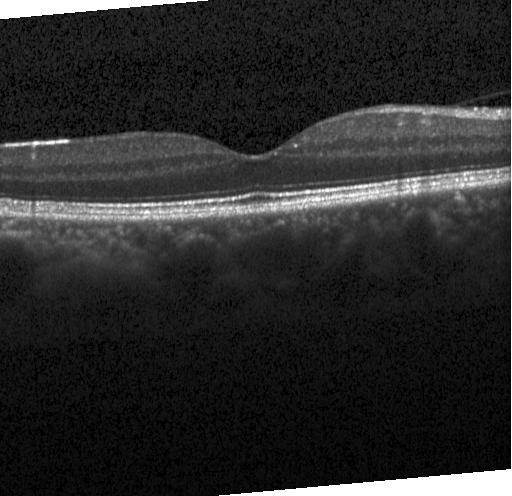 Through the macula, retinal OCT B-scan.
The scan shows no CNV, DME, or drusen.